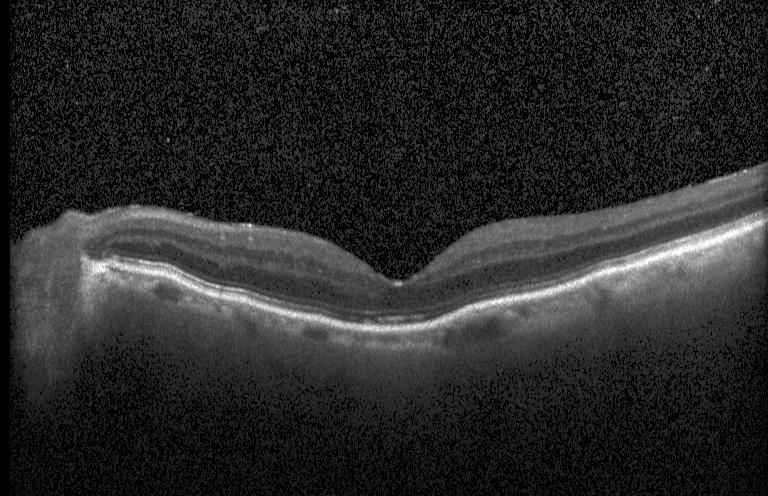 Macular scan · retinal OCT B-scan · spectral-domain OCT · Heidelberg Spectralis. This B-scan demonstrates no choroidal neovascularization, no diabetic macular edema, and no drusen.